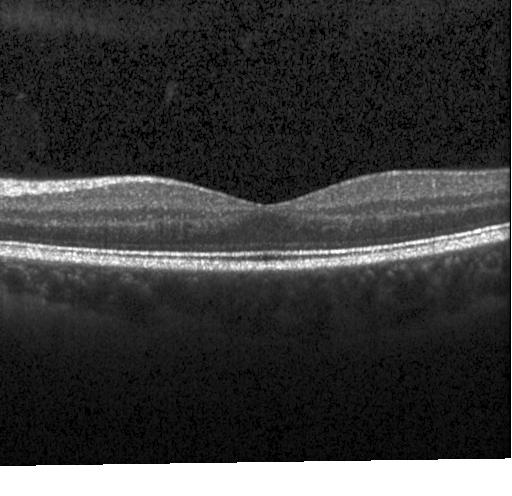 Retinal OCT B-scan. Horizontal scan through the fovea. Heidelberg Spectralis. Spectral-domain OCT — Diagnosis: no choroidal neovascularization, no diabetic macular edema, and no drusen.